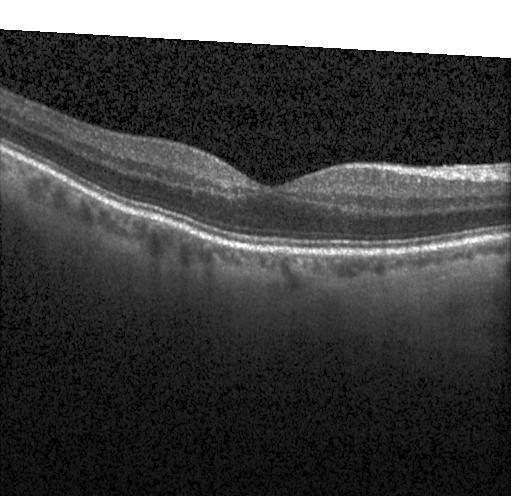

No evidence of choroidal neovascularization, diabetic macular edema, or drusen.